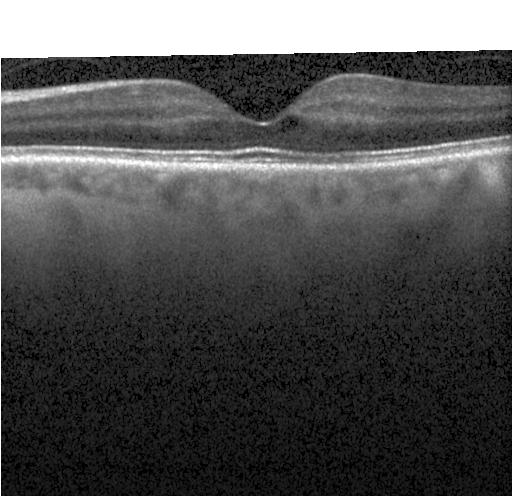

Instrument: Heidelberg Spectralis · retinal OCT cross-section · horizontal scan through the fovea — Macular OCT: diabetic macular edema (DME).